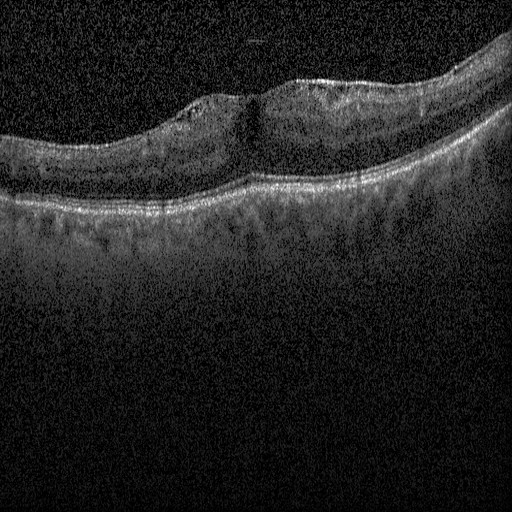

Optical coherence tomography scan.
Dx: diabetic macular edema (DME).